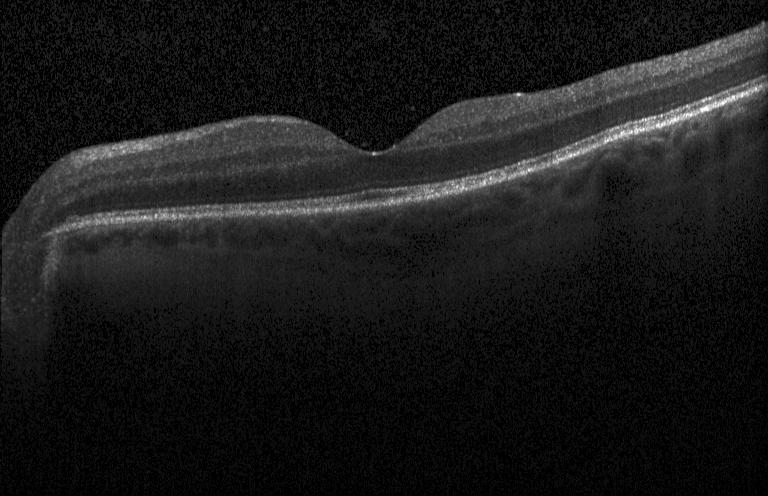

OCT line scan. This B-scan demonstrates no choroidal neovascularization, no diabetic macular edema, and no drusen.